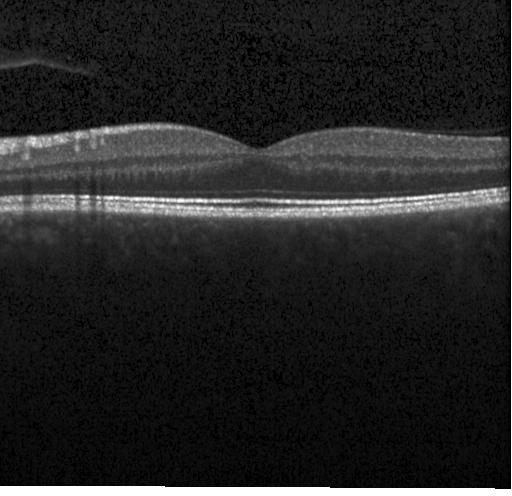

Impression: neither choroidal neovascularization, diabetic macular edema, nor drusen.